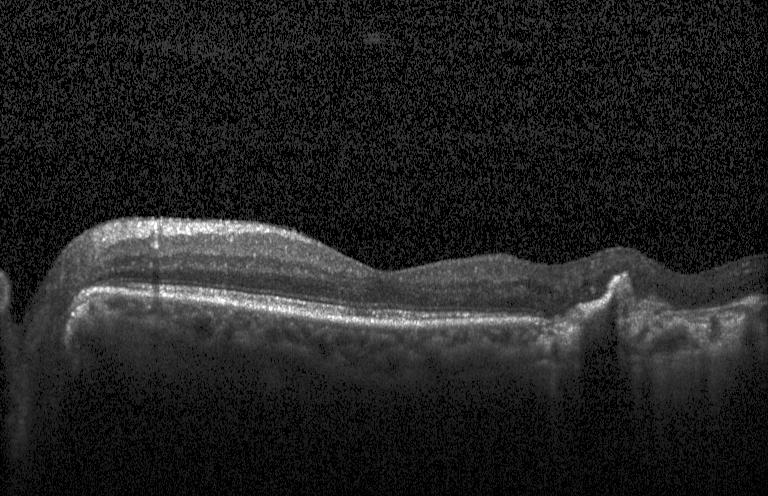

Centered on the fovea; instrument: Heidelberg Spectralis; SD-OCT; OCT line scan — A choroidal neovascular membrane.